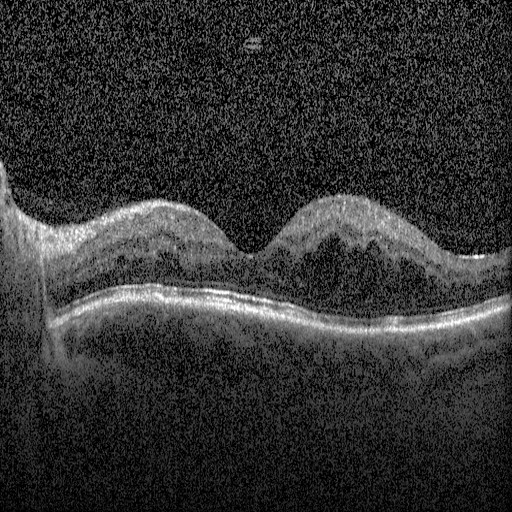
Diagnosis: diabetic macular edema.